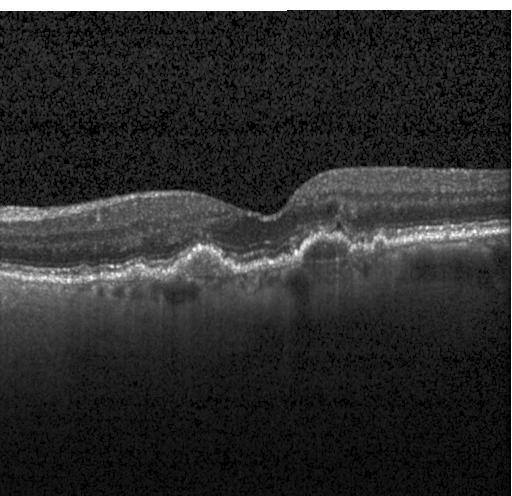

Dx: CNV.